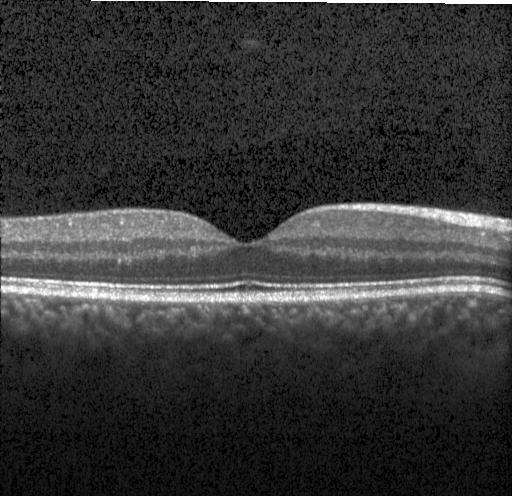

Impression: no evidence of choroidal neovascularization, diabetic macular edema, or drusen.